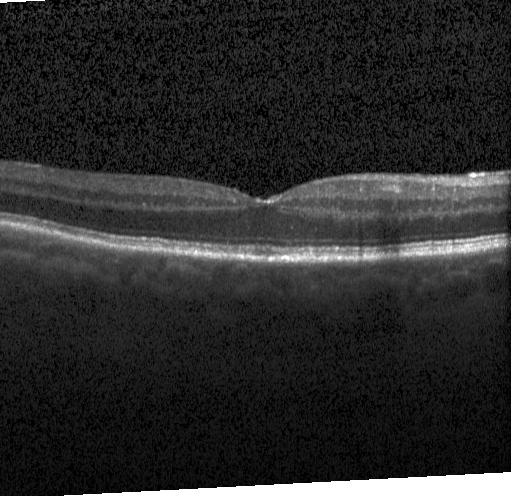
OCT finding: no choroidal neovascularization, no diabetic macular edema, and no drusen.